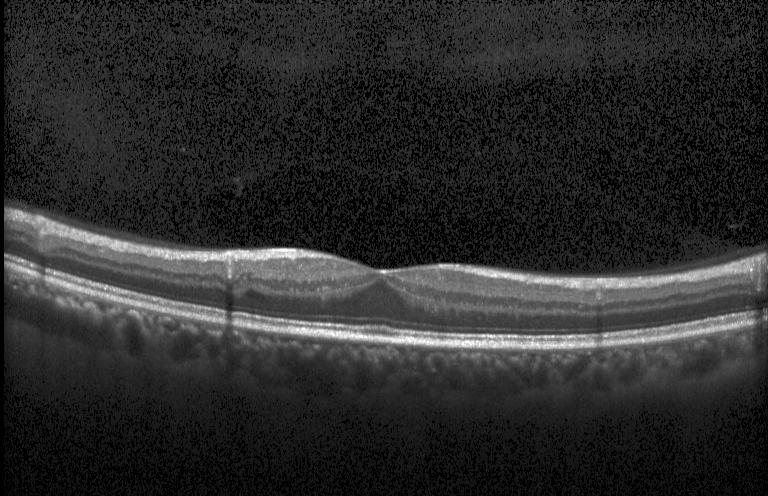 Retinal OCT cross-section · spectral-domain optical coherence tomography
Diagnosis: no choroidal neovascularization, no diabetic macular edema, and no drusen.